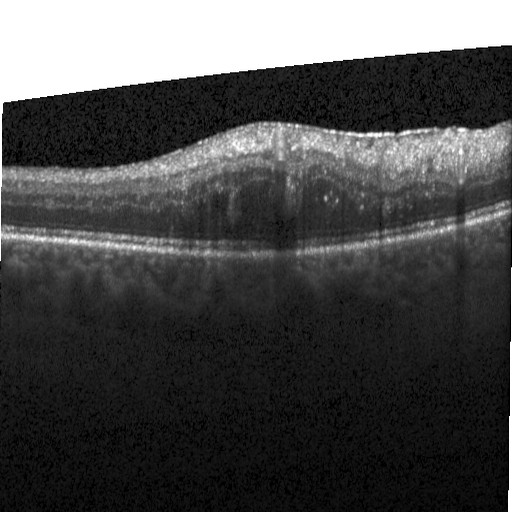
Dx: diabetic macular edema.